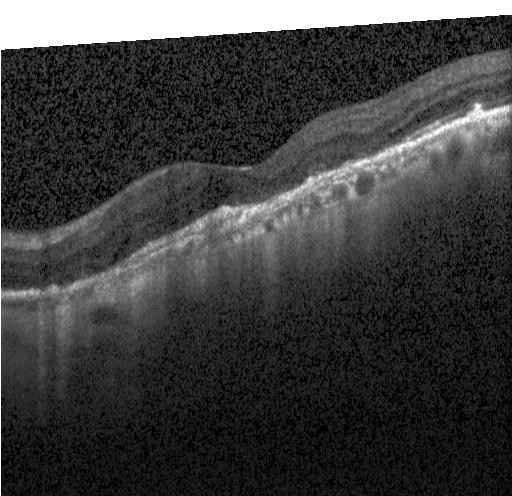 Diagnosis: a choroidal neovascular membrane.